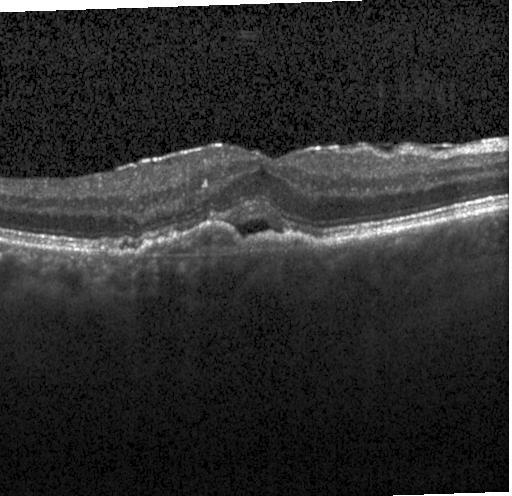 Macular OCT: choroidal neovascularization.